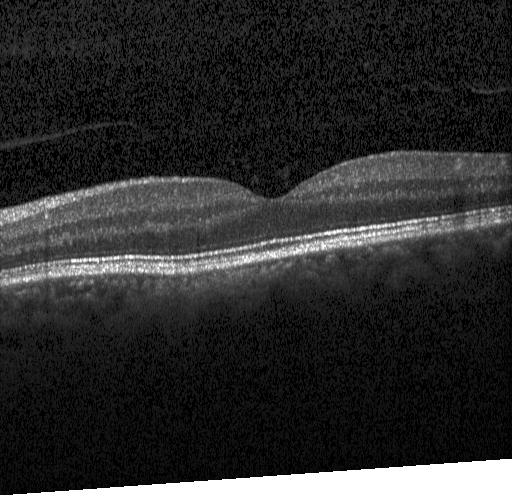
Retinal OCT cross-section
Dx: no evidence of choroidal neovascularization, diabetic macular edema, or drusen.